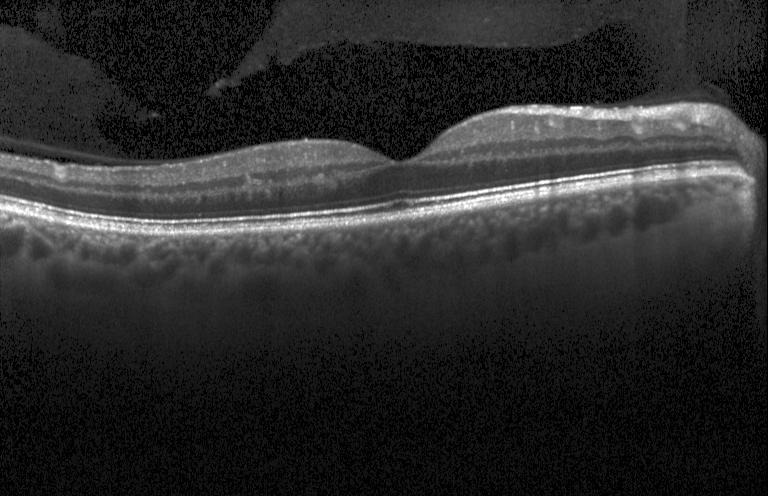 Through the macula; retinal OCT B-scan; SD-OCT; instrument: Heidelberg Spectralis
This B-scan demonstrates neither choroidal neovascularization, diabetic macular edema, nor drusen.